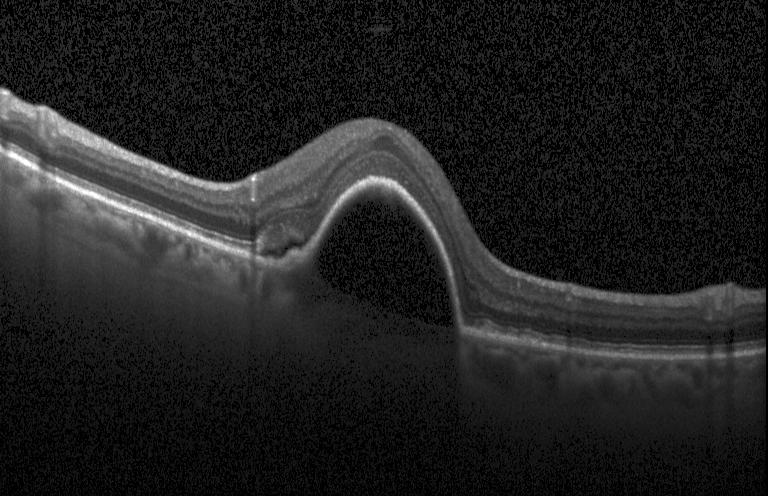

Retinal OCT B-scan
Diagnosis: a choroidal neovascular membrane.